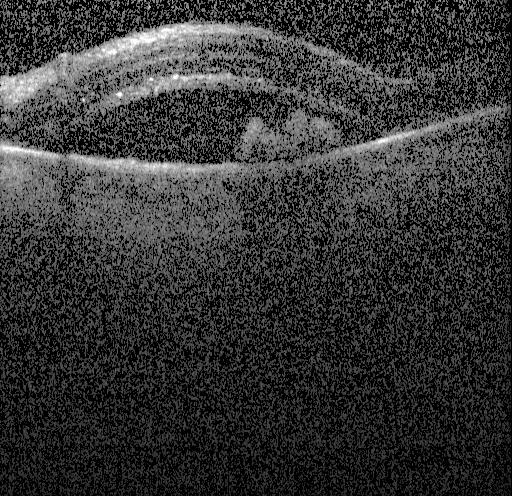

Diagnosis: CNV.